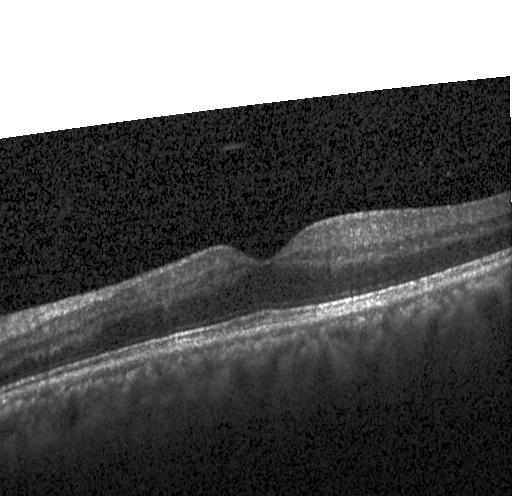

Horizontal scan through the fovea · spectral-domain OCT · OCT line scan — The scan shows neither choroidal neovascularization, diabetic macular edema, nor drusen.